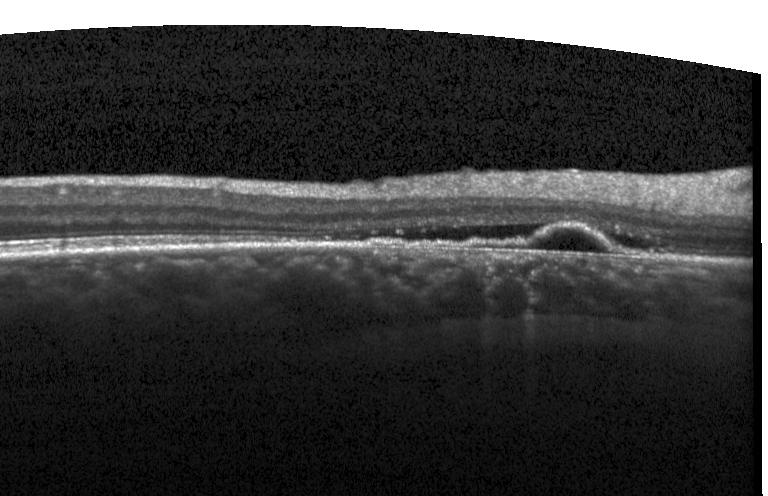

Impression: CNV.